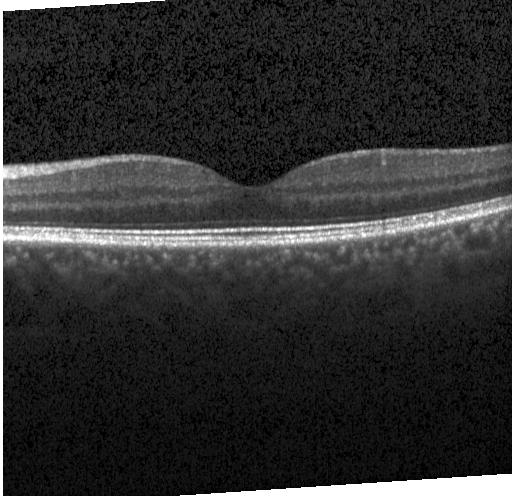 Finding: neither choroidal neovascularization, diabetic macular edema, nor drusen.